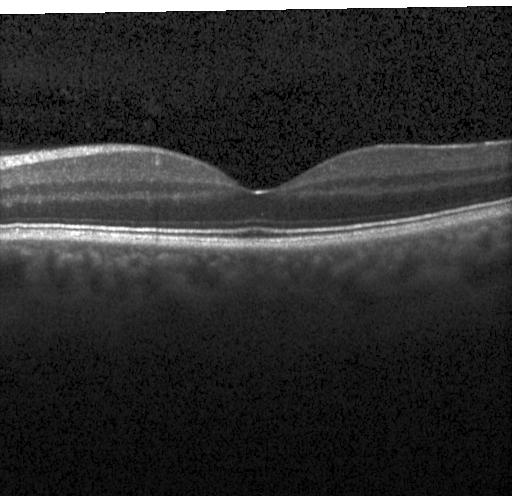 SD-OCT · OCT line scan.
Finding: neither CNV, DME, nor drusen.